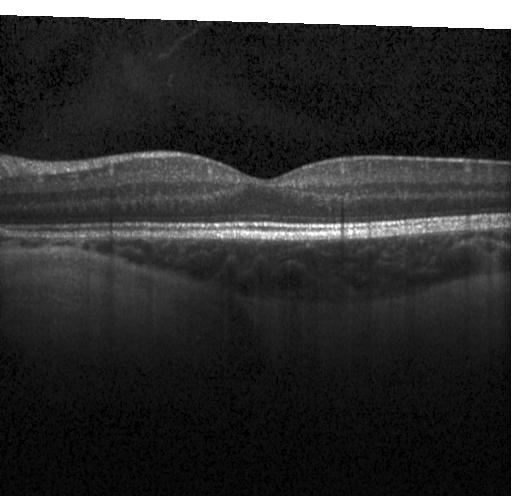

SD-OCT · optical coherence tomography scan · centered on the fovea · Heidelberg Spectralis OCT system. Diagnosis: no CNV, DME, or drusen.